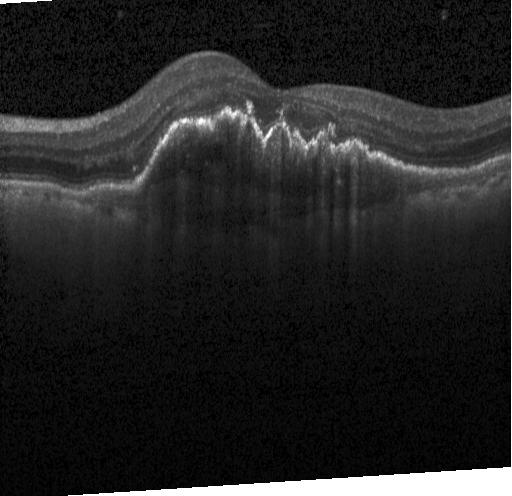
OCT B-scan showing a choroidal neovascular membrane.